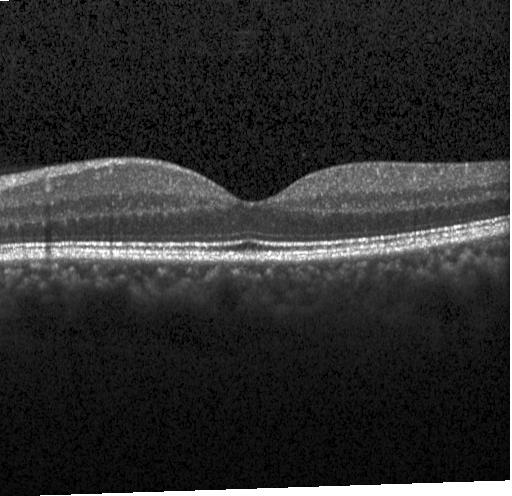
This B-scan demonstrates no evidence of choroidal neovascularization, diabetic macular edema, or drusen.